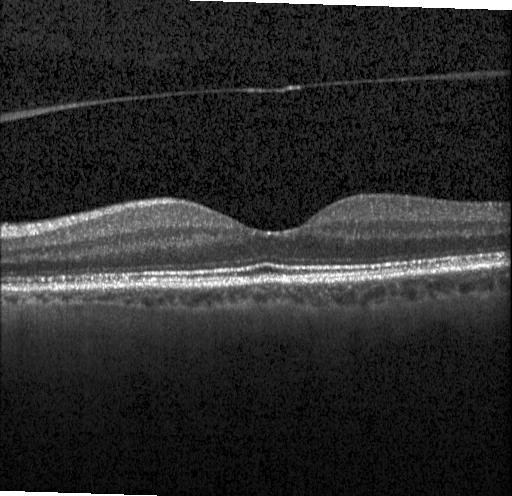
Diagnosis: no evidence of choroidal neovascularization, diabetic macular edema, or drusen.